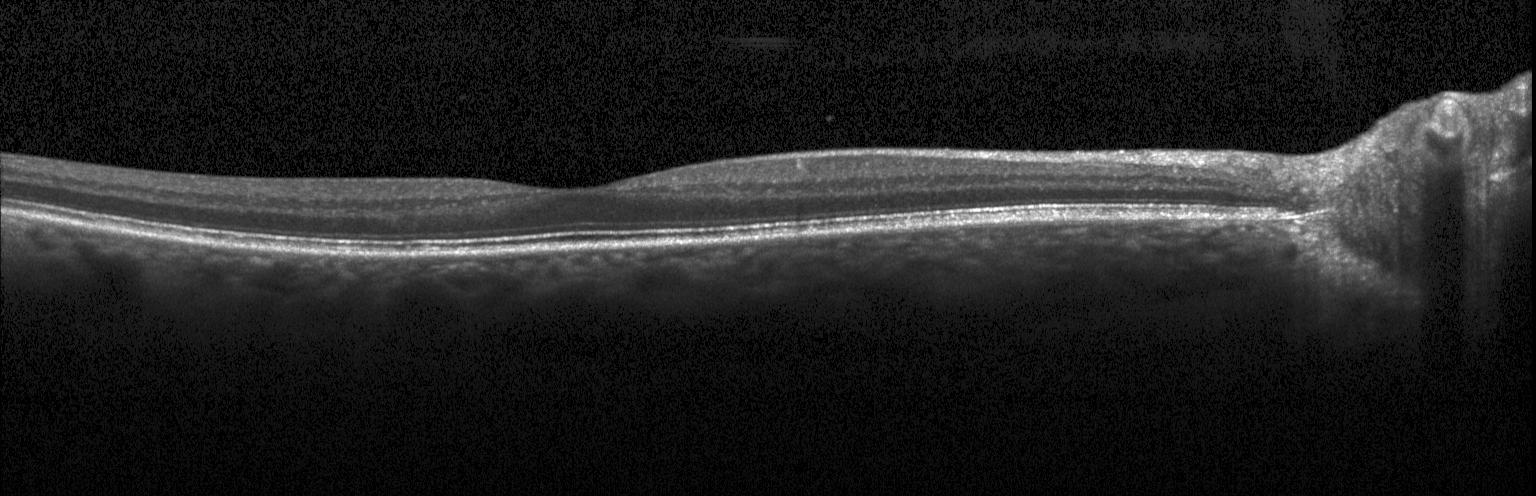 Optical coherence tomography B-scan, spectral-domain OCT.
Finding: no CNV, no DME, and no drusen.